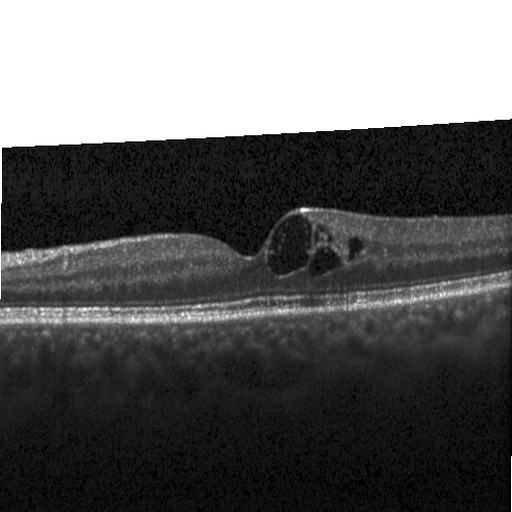
OCT B-scan.
Diabetic macular edema (DME).